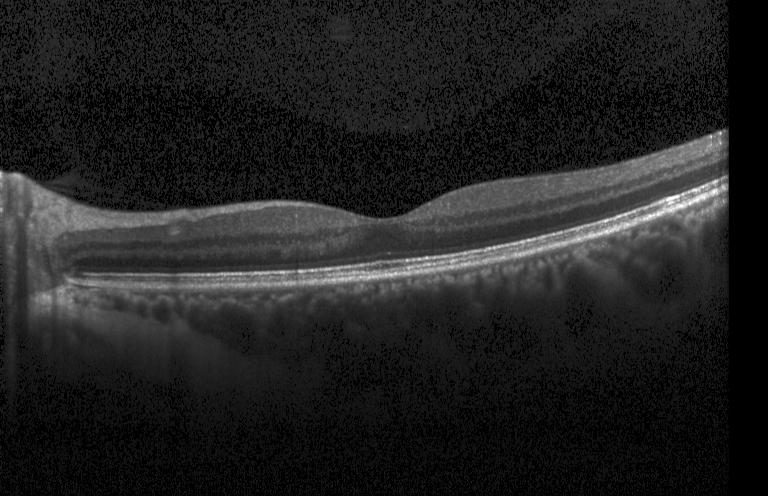
Optical coherence tomography B-scan, Heidelberg Spectralis — Impression: no choroidal neovascularization, no diabetic macular edema, and no drusen.